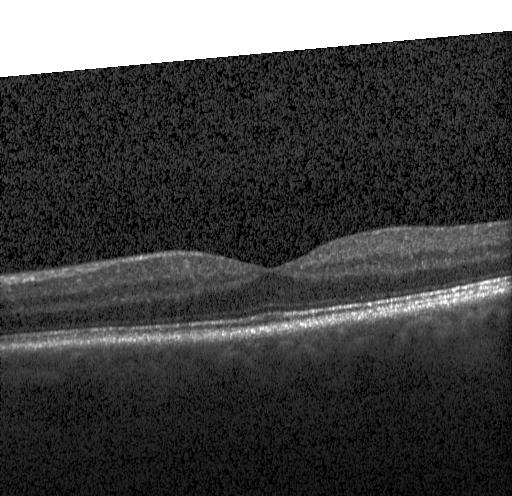
Macular OCT demonstrating no choroidal neovascularization, diabetic macular edema, or drusen.